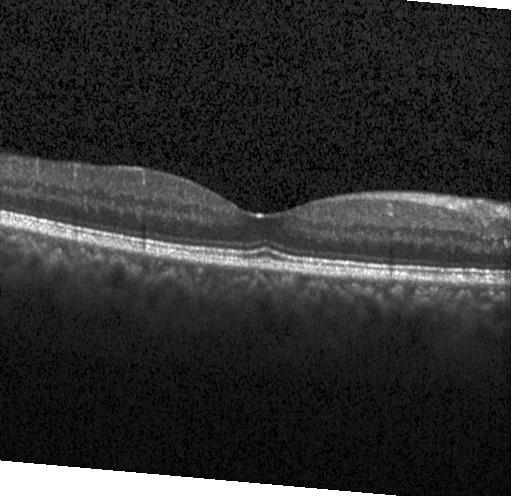 Horizontal scan through the fovea; optical coherence tomography B-scan; instrument: Heidelberg Spectralis — Macular OCT: no CNV, DME, or drusen.